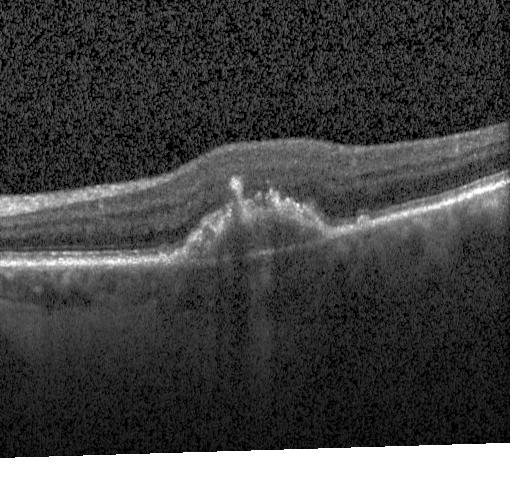
OCT B-scan — Impression: choroidal neovascularization.